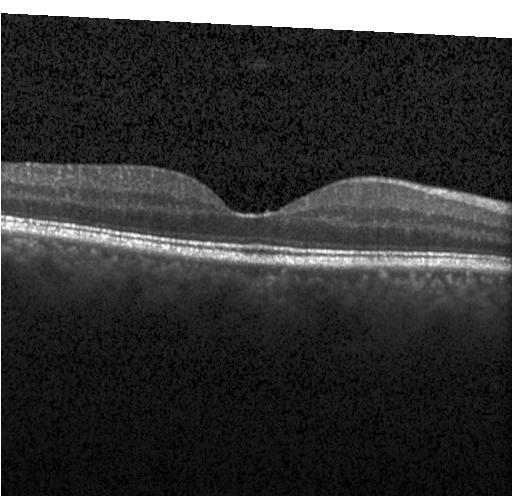

Diagnosis: no CNV, DME, or drusen.